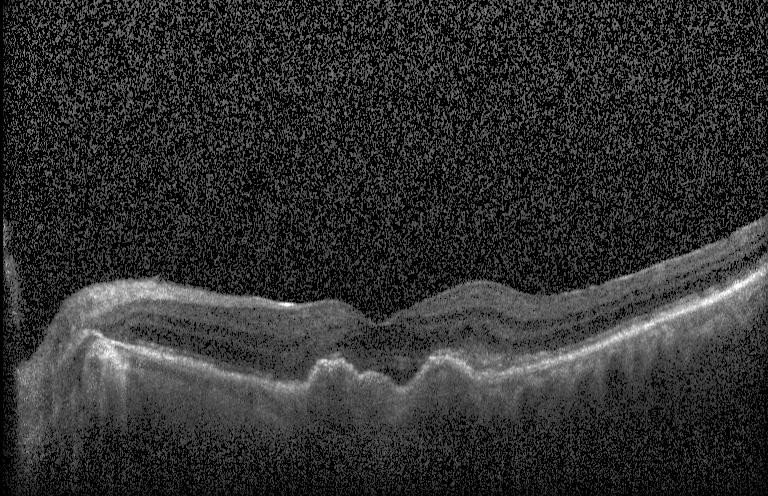

Centered on the fovea; OCT B-scan — Choroidal neovascularization (CNV).